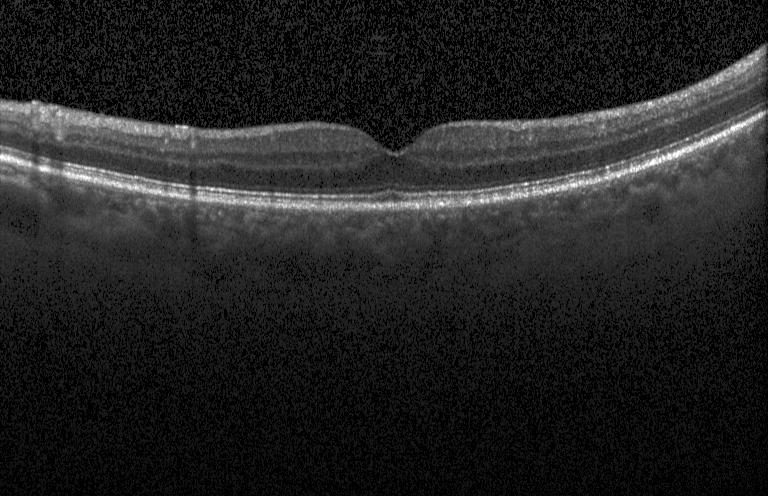
Macular OCT demonstrating no evidence of choroidal neovascularization, diabetic macular edema, or drusen.